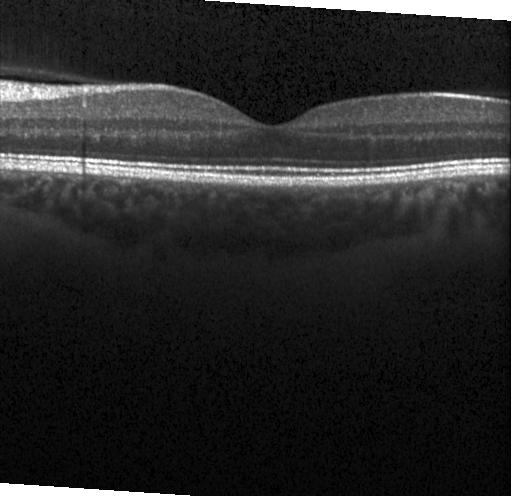

Spectral-domain OCT · optical coherence tomography scan · horizontal scan through the fovea — Finding: no choroidal neovascularization, no diabetic macular edema, and no drusen.